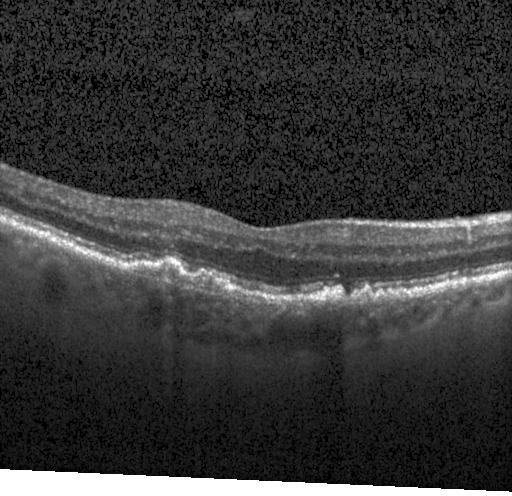
Retinal OCT cross-section, macular scan. OCT finding: choroidal neovascularization.